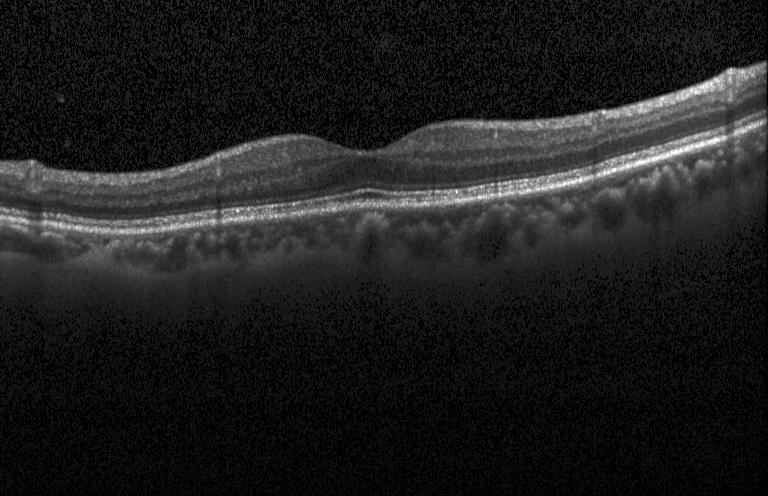

Retinal OCT cross-section — Impression: neither choroidal neovascularization, diabetic macular edema, nor drusen.